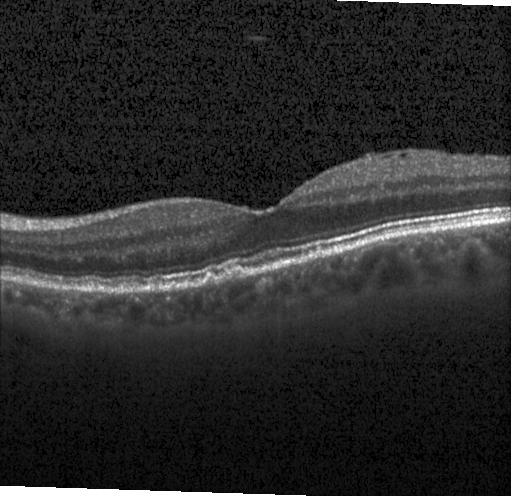
OCT finding: drusen.